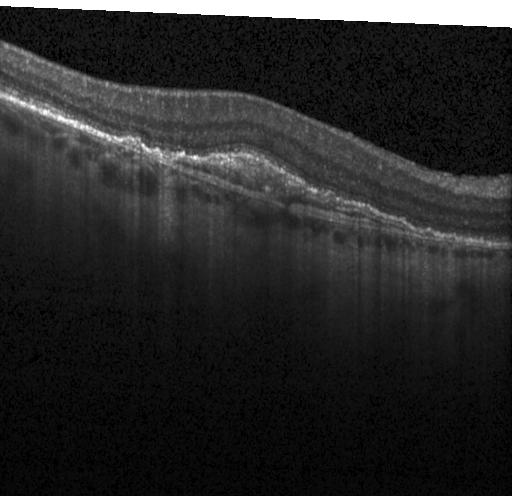 Heidelberg Spectralis, optical coherence tomography scan, SD-OCT.
Diagnosis: a choroidal neovascular membrane.